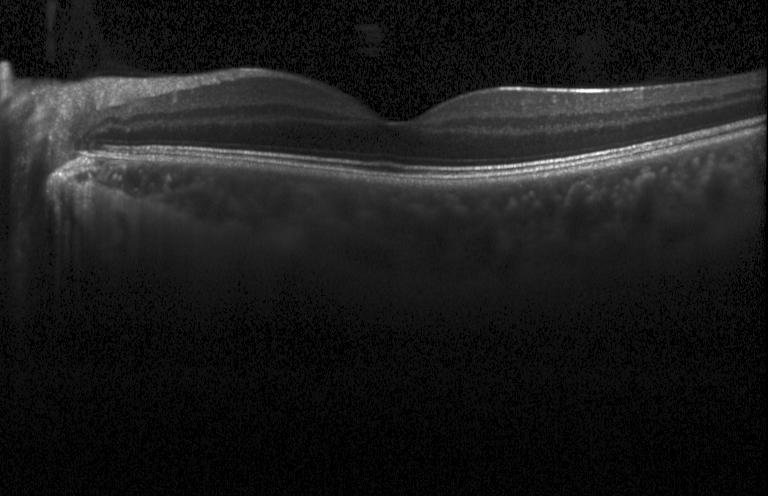 No evidence of choroidal neovascularization, diabetic macular edema, or drusen.